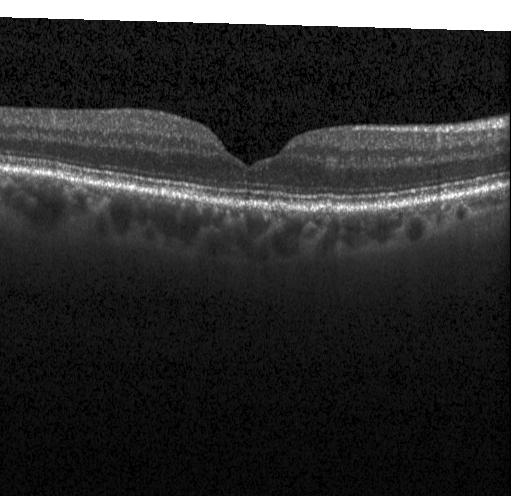
Acquired on a Heidelberg Spectralis, SD-OCT, OCT line scan.
Impression: no choroidal neovascularization, diabetic macular edema, or drusen.